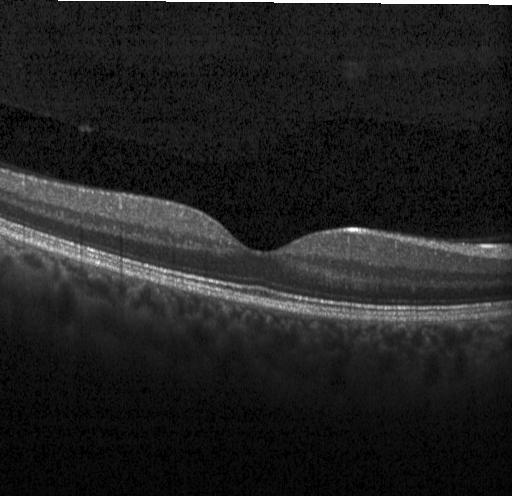

Impression: no choroidal neovascularization, diabetic macular edema, or drusen.